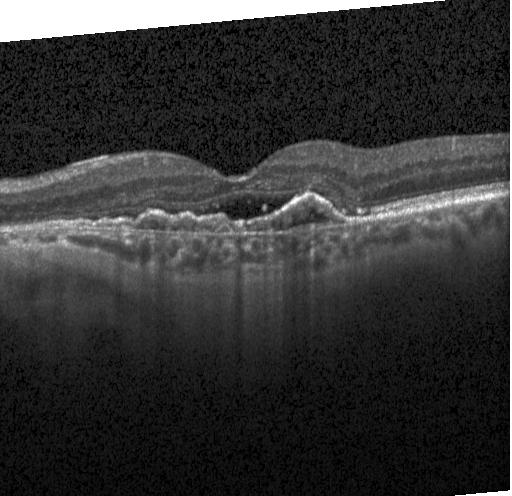 Spectral-domain OCT; optical coherence tomography scan; fovea-centered; Heidelberg Spectralis OCT system
Impression: a choroidal neovascular membrane.